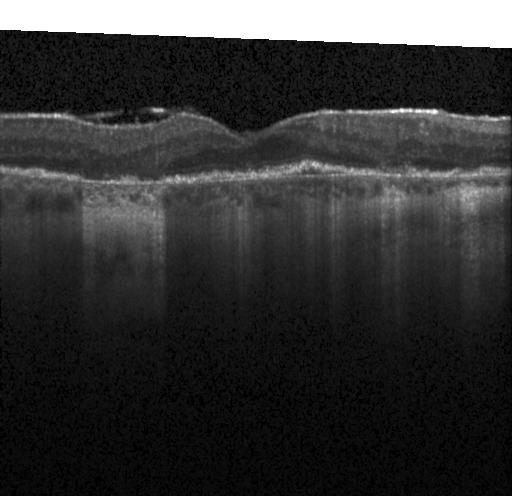
SD-OCT · OCT line scan · fovea-centered · Heidelberg Spectralis.
Finding: choroidal neovascularization (CNV).